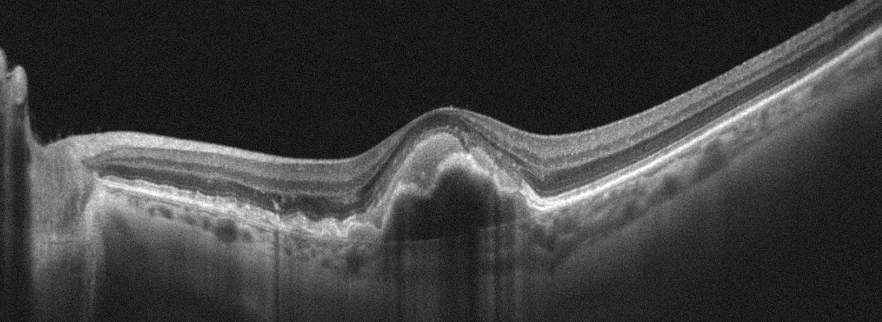 Retinal OCT B-scan. Dx: age-related macular degeneration (AMD).